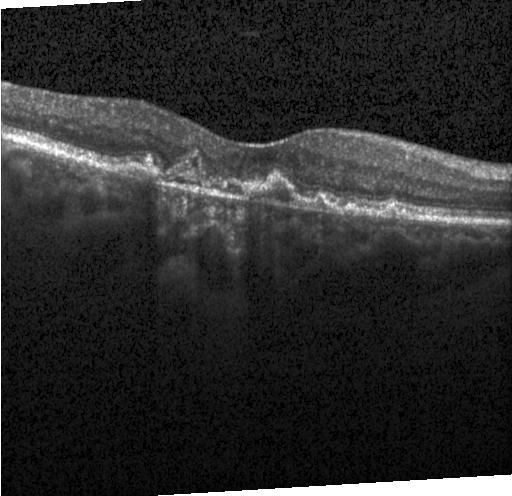
OCT B-scan showing CNV.